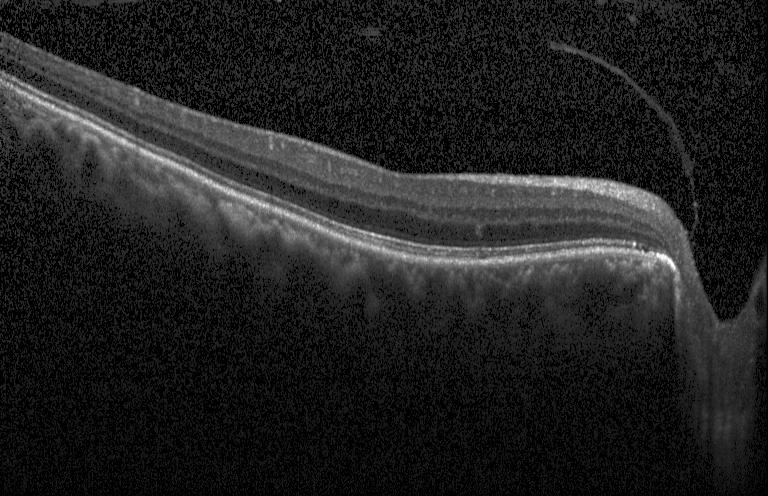

Optical coherence tomography scan. Spectral-domain optical coherence tomography. Horizontal scan through the fovea. Heidelberg Spectralis OCT system. Neither choroidal neovascularization, diabetic macular edema, nor drusen.